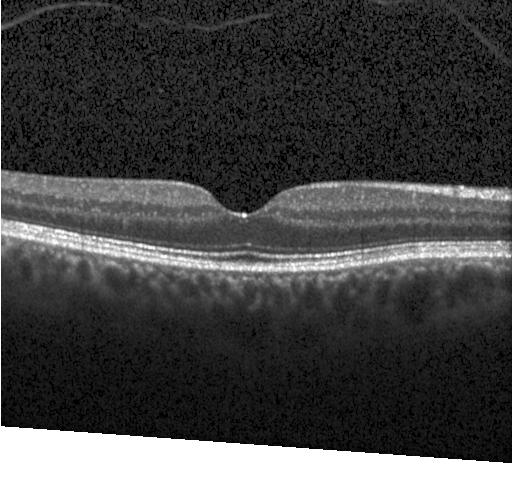
Spectral-domain OCT · OCT line scan
Diagnosis: no evidence of CNV, DME, or drusen.